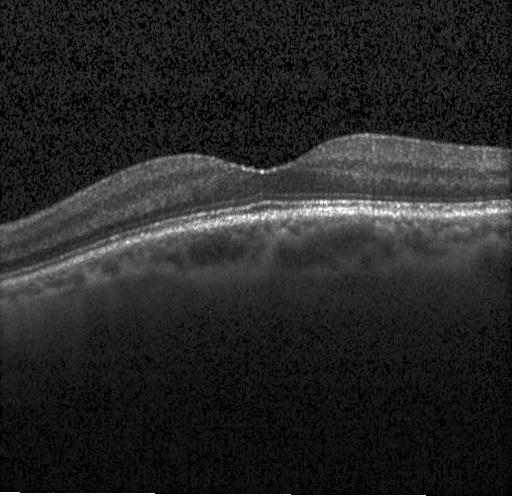

Optical coherence tomography scan; instrument: Heidelberg Spectralis; through the macula.
Impression: no choroidal neovascularization, no diabetic macular edema, and no drusen.